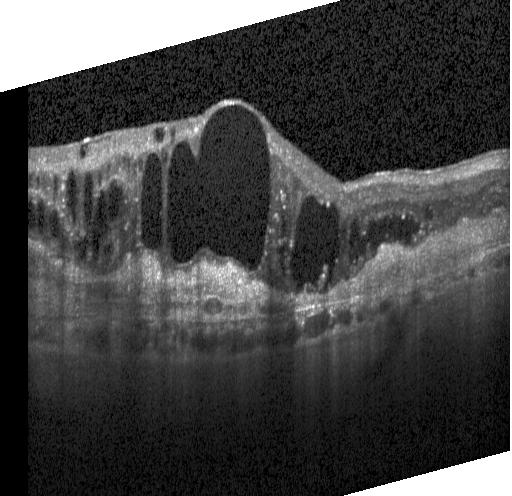 Optical coherence tomography B-scan. Assessment: CNV.